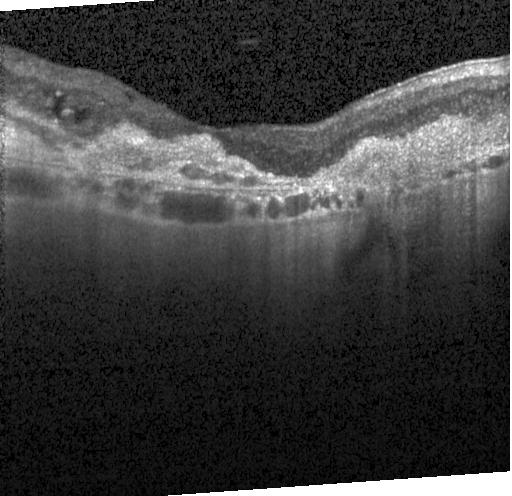

Centered on the fovea; SD-OCT; OCT B-scan; Heidelberg Spectralis OCT system. Finding: a choroidal neovascular membrane.